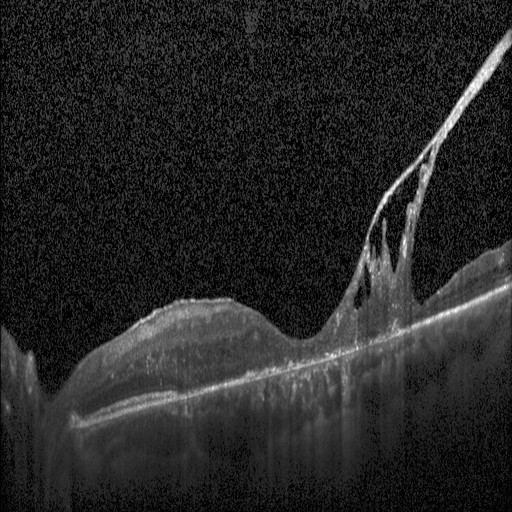

Optical coherence tomography scan · instrument: Heidelberg Spectralis · through the macula — Assessment: diabetic macular edema.